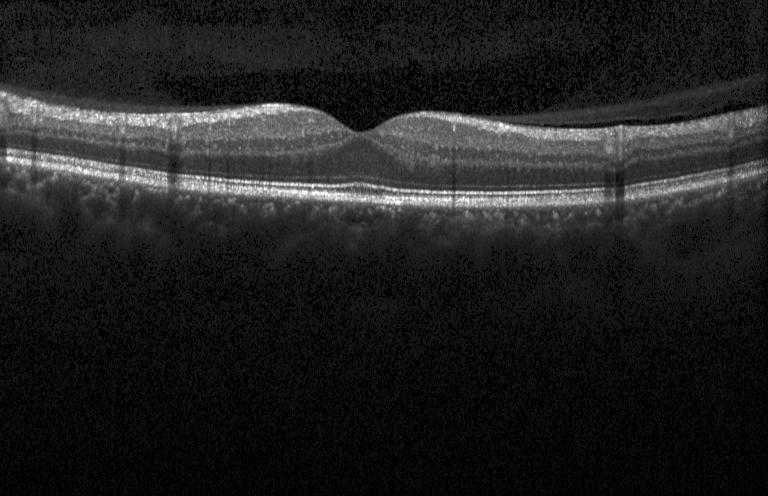

Dx: no CNV, no DME, and no drusen.